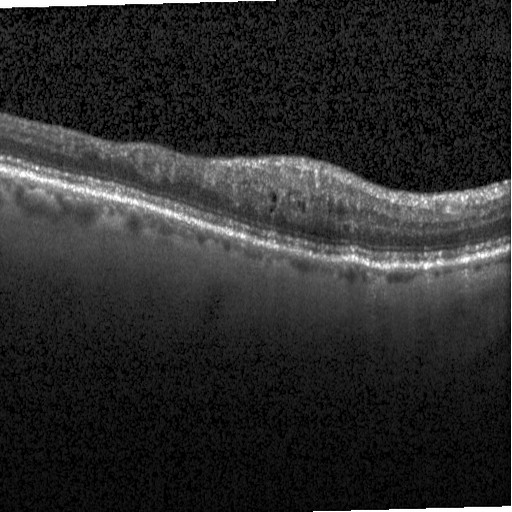 Macular OCT: diabetic macular edema (DME).